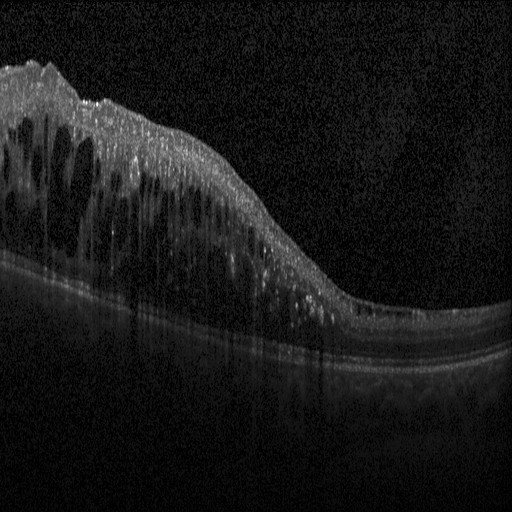
Instrument: Heidelberg Spectralis; fovea-centered; optical coherence tomography scan.
Diagnosis: diabetic macular edema.